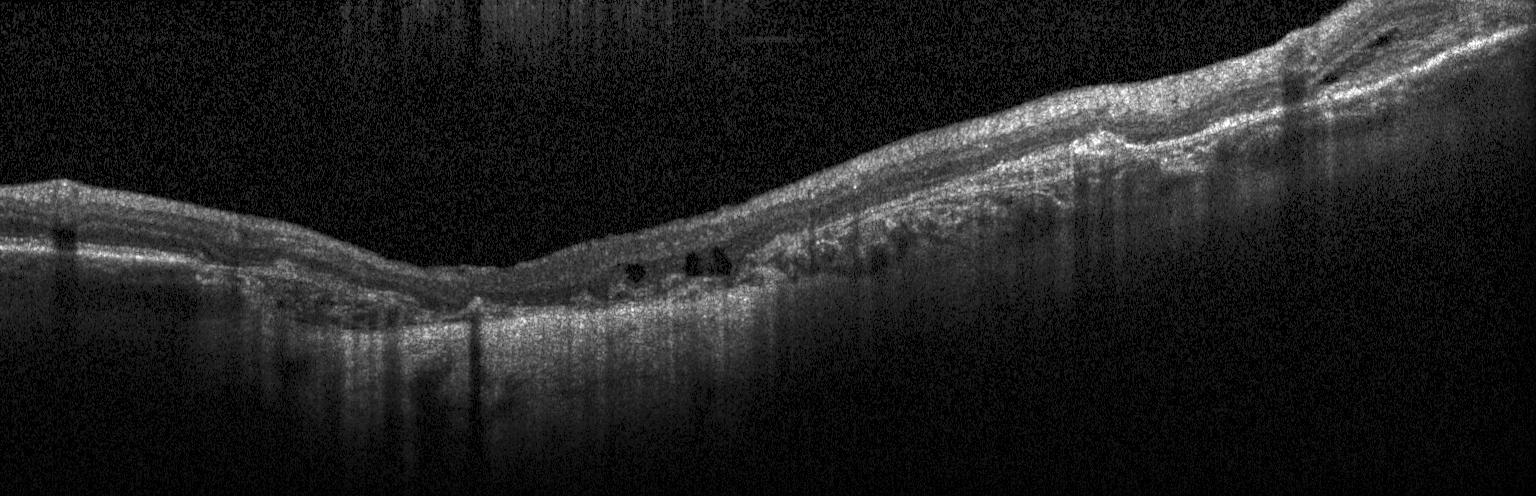
Through the macula; OCT B-scan; Heidelberg Spectralis. The scan shows choroidal neovascularization (CNV).